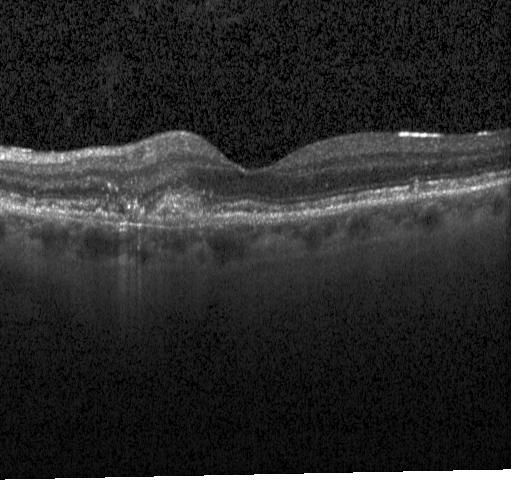
Through the macula; optical coherence tomography scan; spectral-domain OCT; Heidelberg Spectralis
Assessment: a choroidal neovascular membrane.